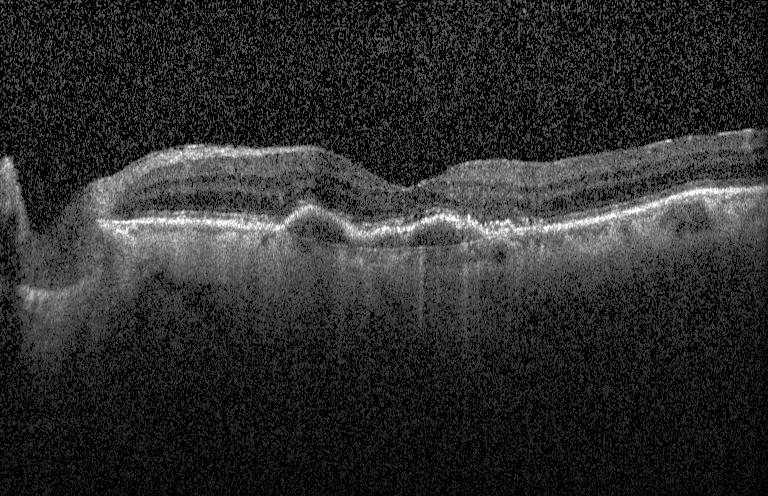

Optical coherence tomography scan — OCT finding: a choroidal neovascular membrane.